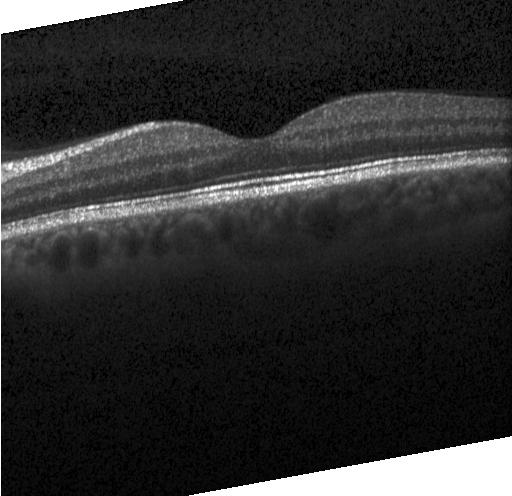 Impression: neither CNV, DME, nor drusen.